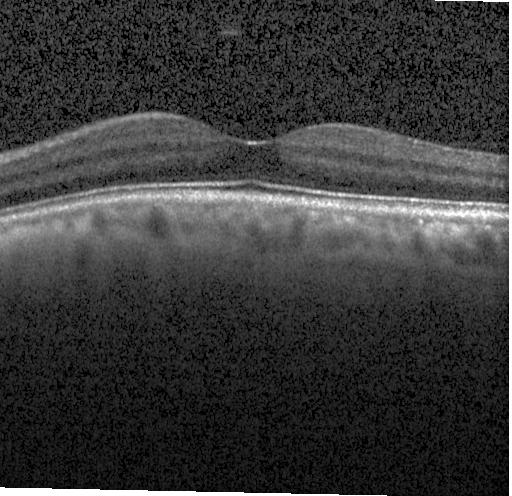 Diagnosis: no choroidal neovascularization, diabetic macular edema, or drusen.